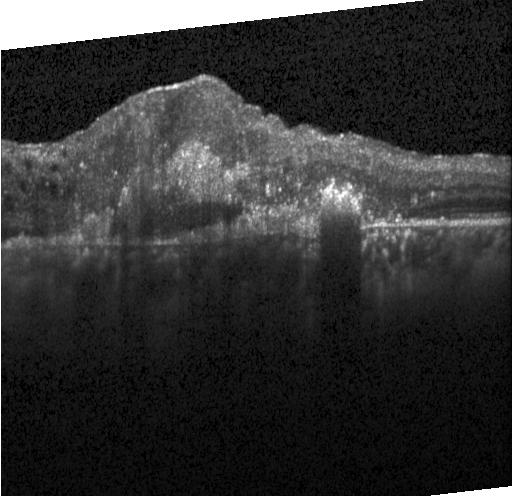 Spectral-domain optical coherence tomography; macular scan; optical coherence tomography scan — A choroidal neovascular membrane.